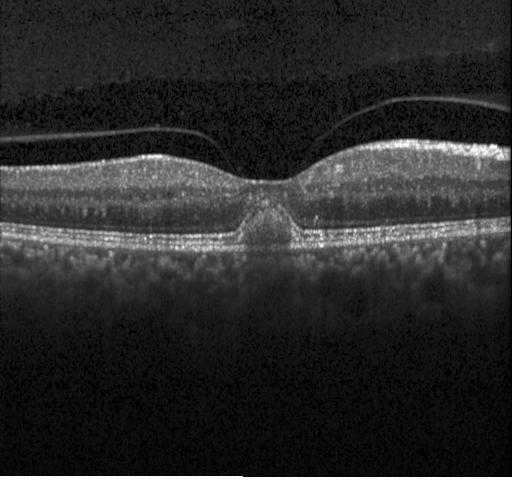
Macular scan; optical coherence tomography B-scan
Impression: a choroidal neovascular membrane.